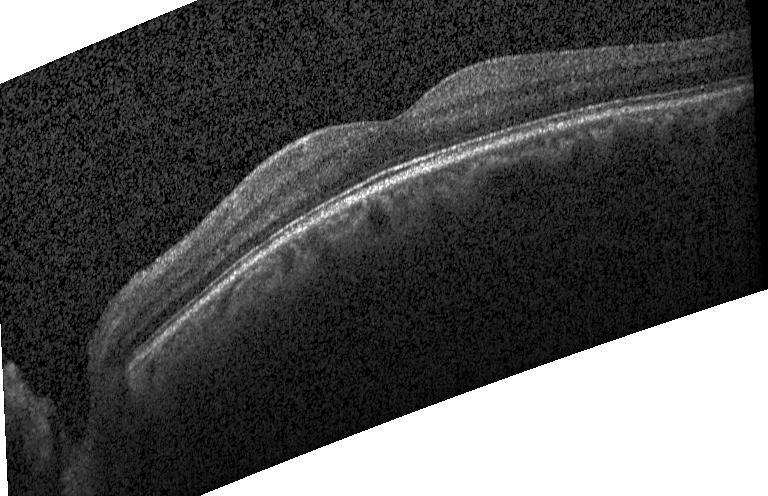

Assessment: no choroidal neovascularization, no diabetic macular edema, and no drusen.